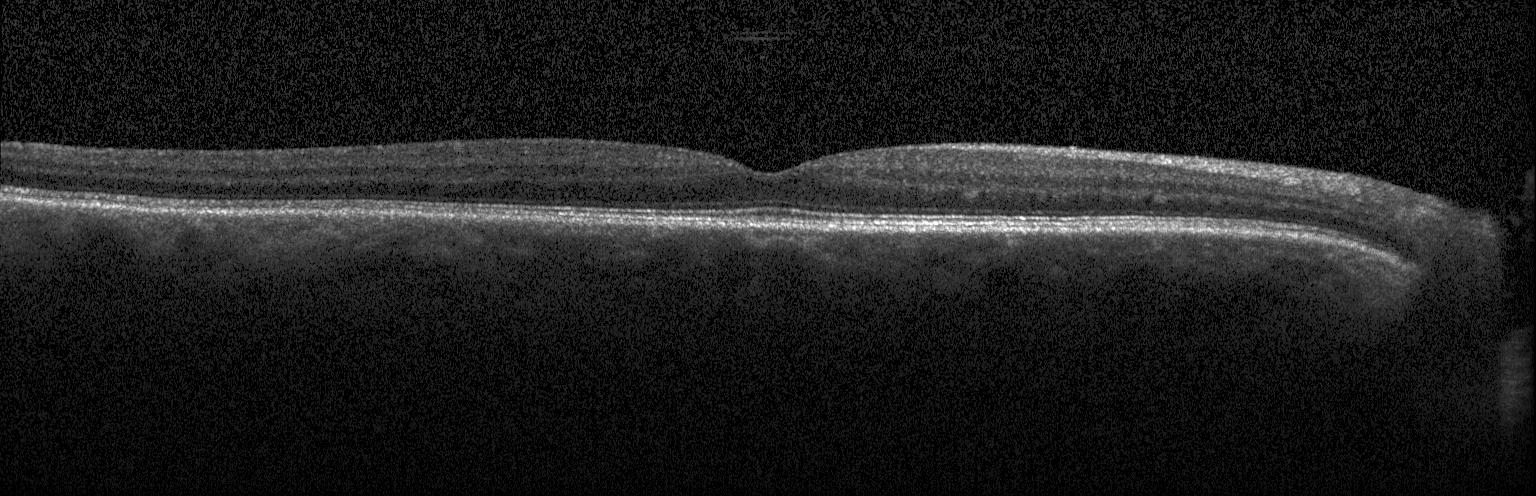

OCT finding: no choroidal neovascularization, no diabetic macular edema, and no drusen.